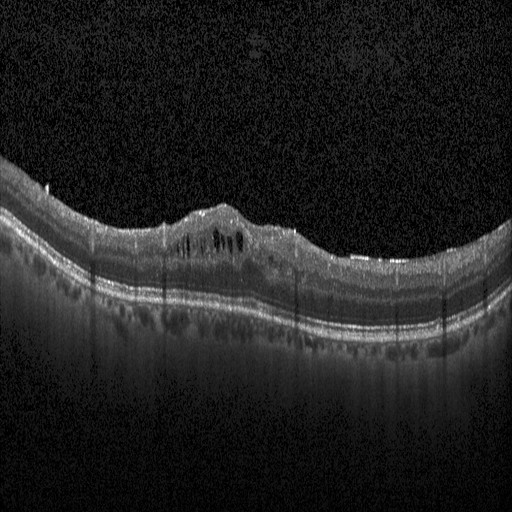 Assessment: diabetic macular edema (DME).